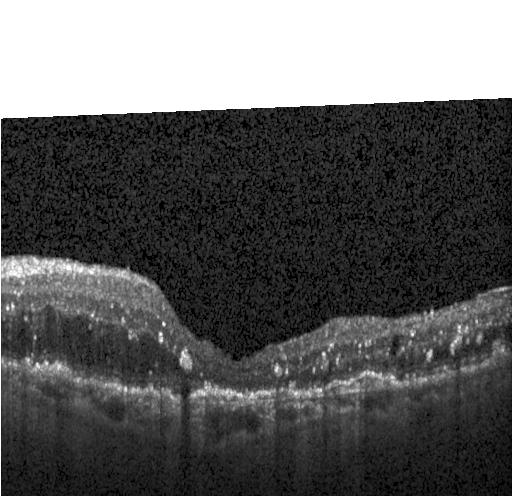
OCT finding: a choroidal neovascular membrane.